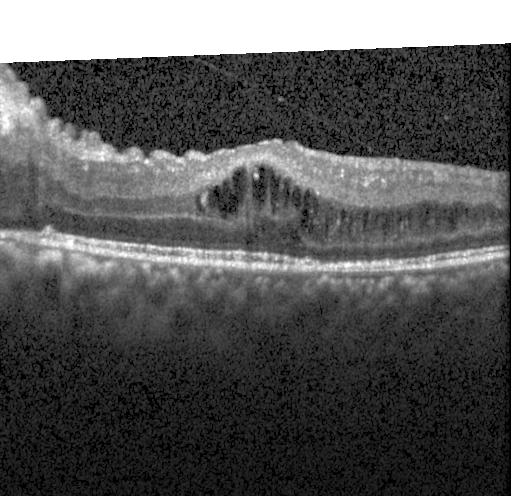
Optical coherence tomography B-scan · SD-OCT · Heidelberg Spectralis OCT system — Impression: diabetic macular edema (DME).